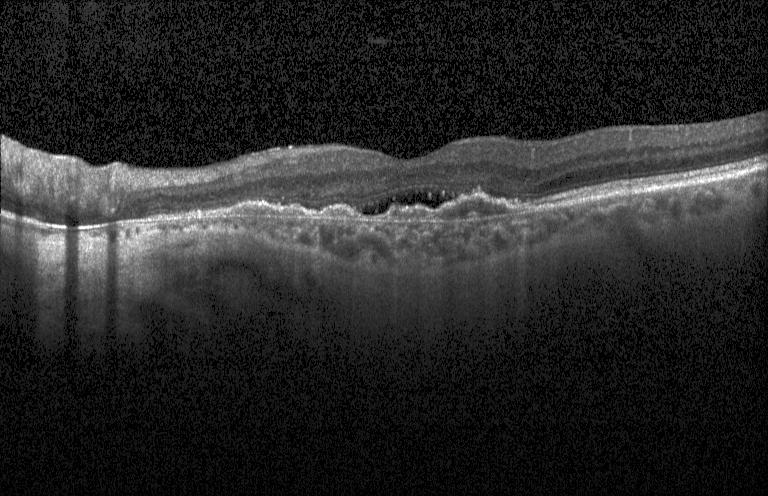

Macular OCT demonstrating choroidal neovascularization.